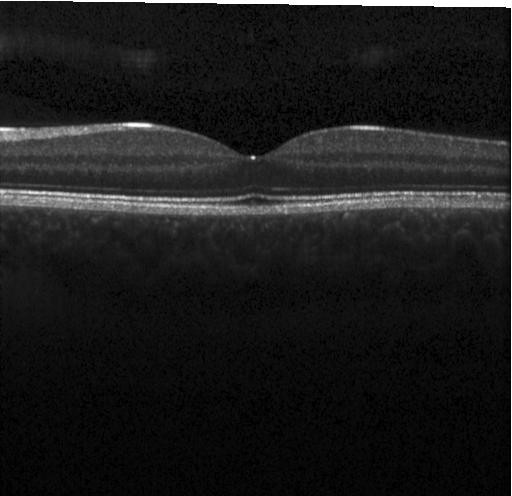

Dx: no choroidal neovascularization, diabetic macular edema, or drusen.